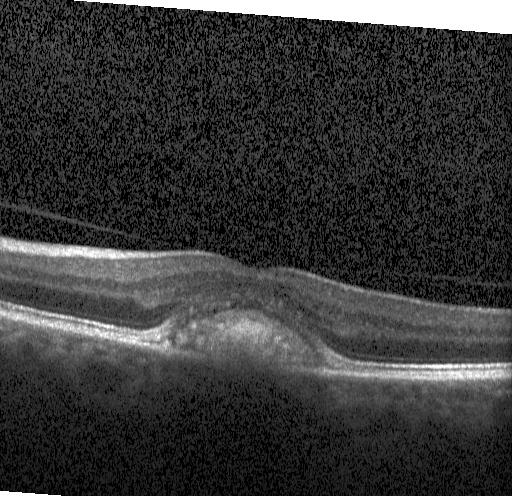 Optical coherence tomography scan, spectral-domain OCT, instrument: Heidelberg Spectralis.
The scan shows CNV.